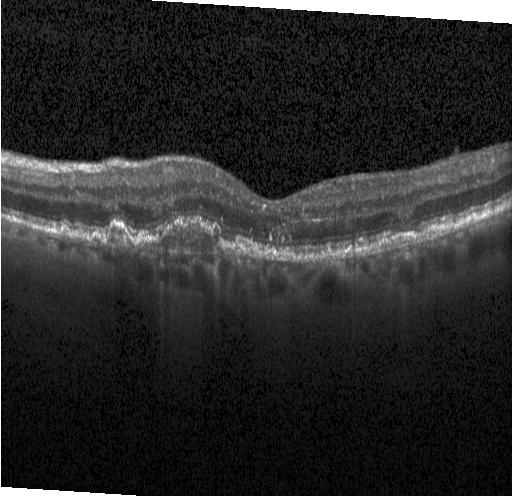

Retinal OCT cross-section. Horizontal scan through the fovea — Diagnosis: a choroidal neovascular membrane.